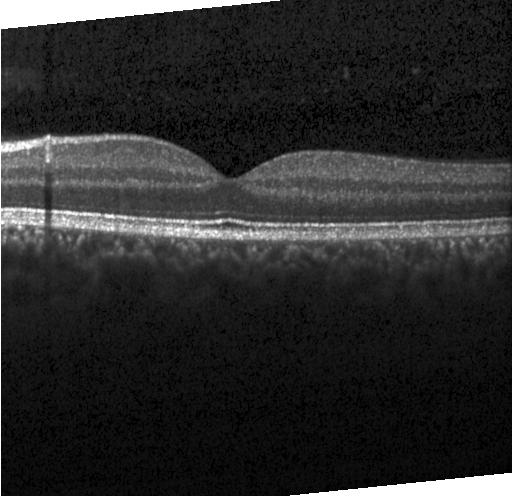 Retinal OCT cross-section showing no choroidal neovascularization, no diabetic macular edema, and no drusen.